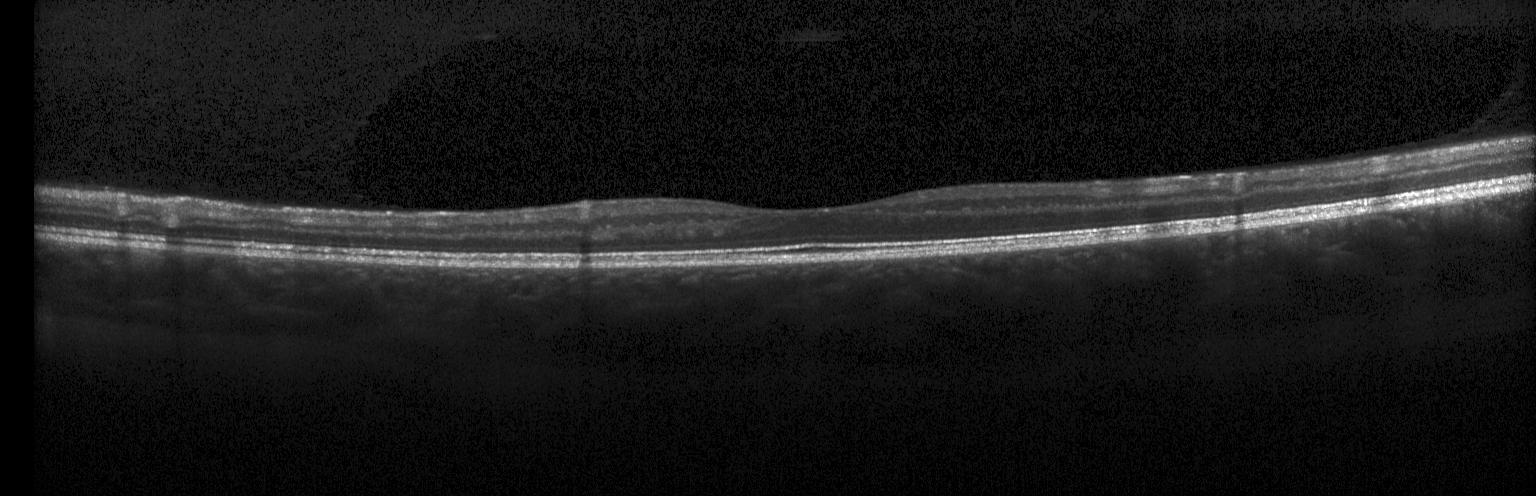
Fovea-centered, OCT line scan
This B-scan demonstrates no choroidal neovascularization, diabetic macular edema, or drusen.